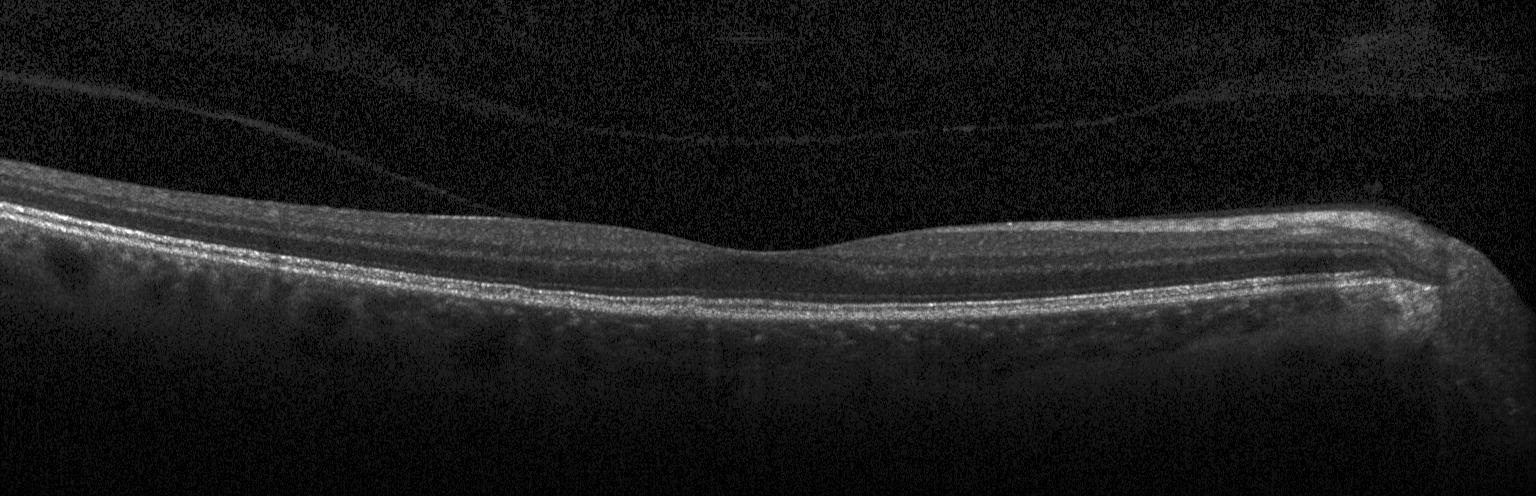

Impression: no choroidal neovascularization, no diabetic macular edema, and no drusen.